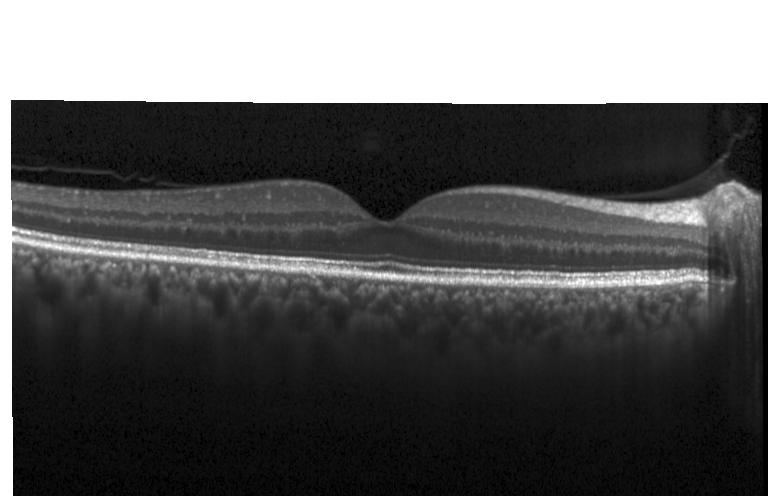 Through the macula, OCT line scan.
OCT finding: neither CNV, DME, nor drusen.